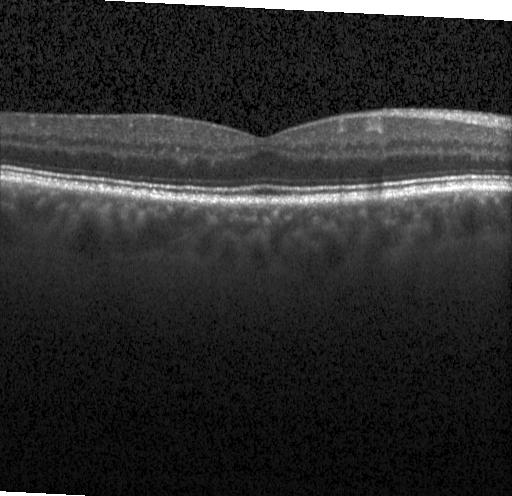 SD-OCT. OCT line scan. Centered on the fovea. Heidelberg Spectralis OCT system. This B-scan demonstrates no choroidal neovascularization, no diabetic macular edema, and no drusen.